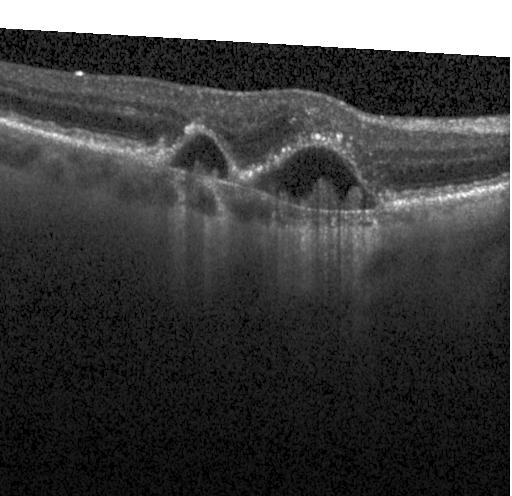

Fovea-centered. Heidelberg Spectralis OCT system. Optical coherence tomography B-scan
Assessment: a choroidal neovascular membrane.